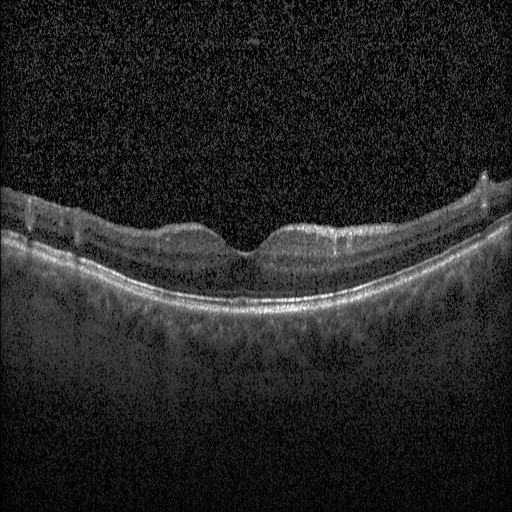

Acquired on a Heidelberg Spectralis · SD-OCT · OCT B-scan — Impression: diabetic macular edema.